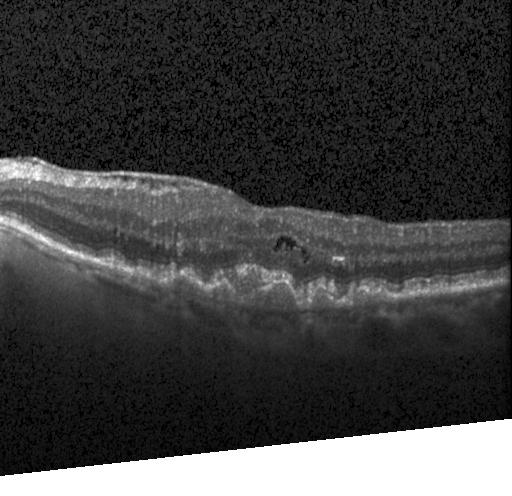 Optical coherence tomography B-scan
Dx: a choroidal neovascular membrane.